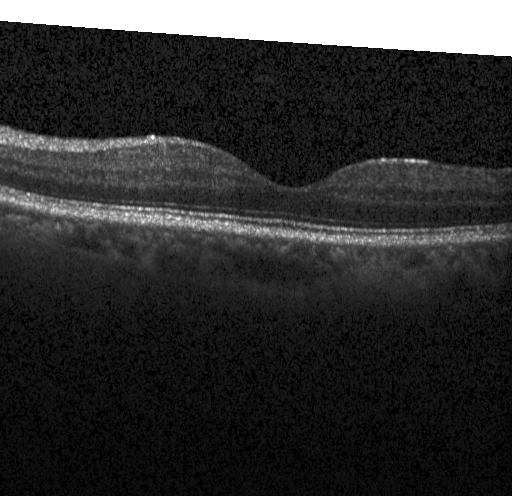

Horizontal scan through the fovea · optical coherence tomography B-scan — No choroidal neovascularization, diabetic macular edema, or drusen.